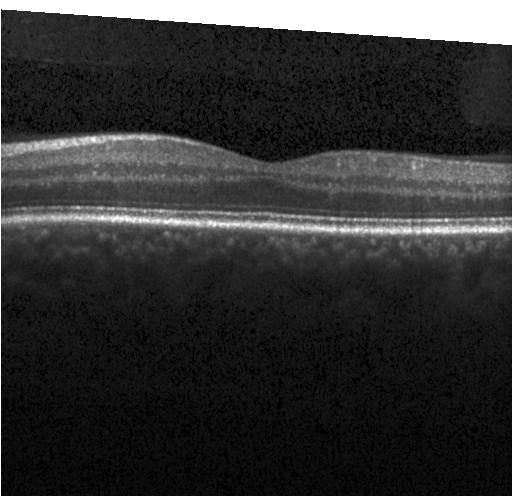 OCT line scan.
Finding: no CNV, DME, or drusen.